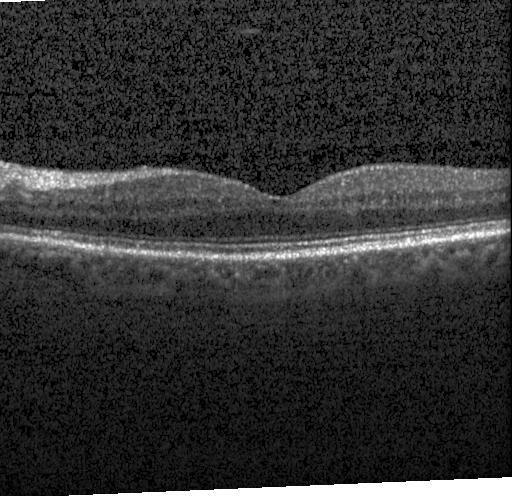 Finding: neither choroidal neovascularization, diabetic macular edema, nor drusen.